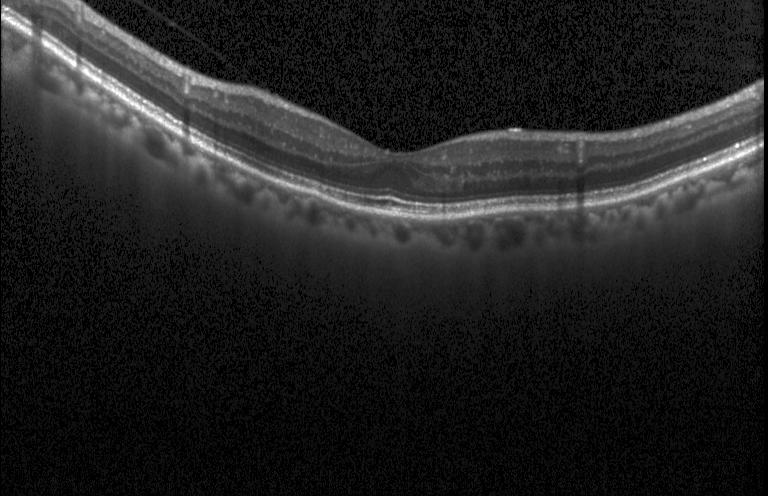 The scan shows no CNV, DME, or drusen.